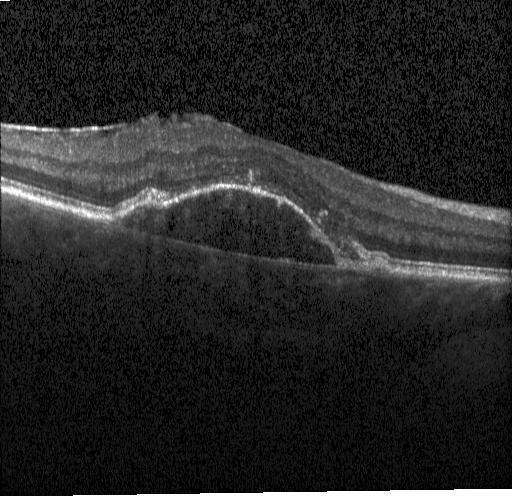

Impression: choroidal neovascularization.